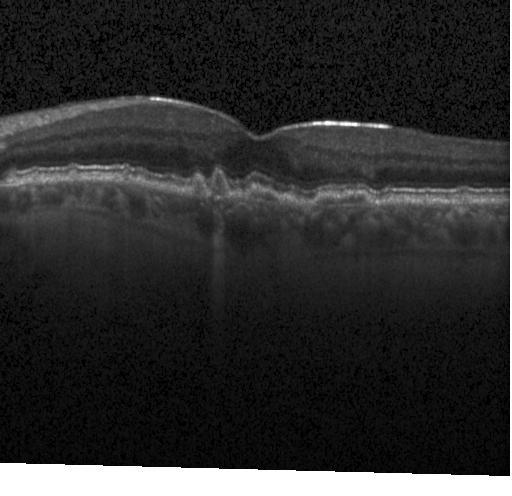 Diagnosis: sub-RPE drusenoid deposits.